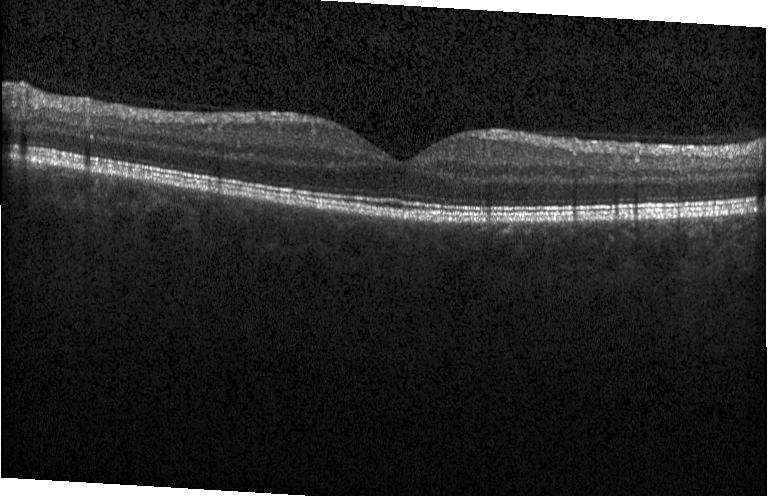 Optical coherence tomography B-scan; Heidelberg Spectralis.
OCT finding: no choroidal neovascularization, no diabetic macular edema, and no drusen.